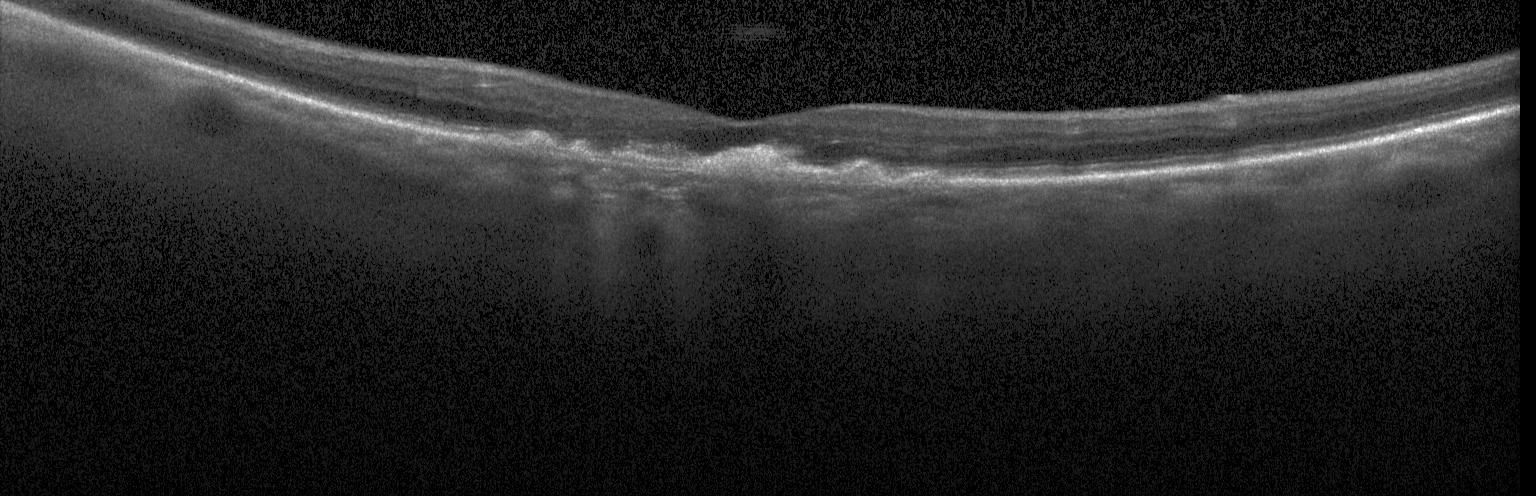
OCT B-scan; SD-OCT. The scan shows a choroidal neovascular membrane.